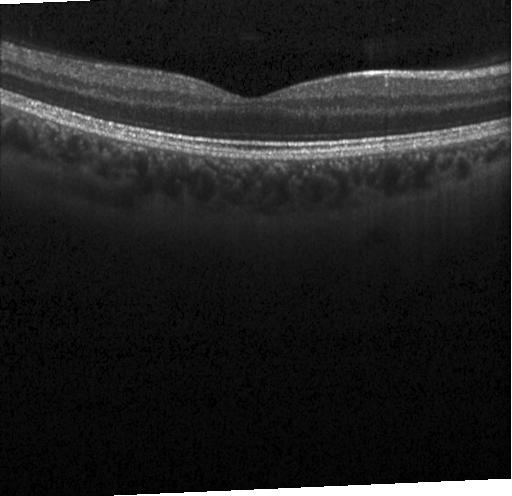

This B-scan demonstrates neither choroidal neovascularization, diabetic macular edema, nor drusen.